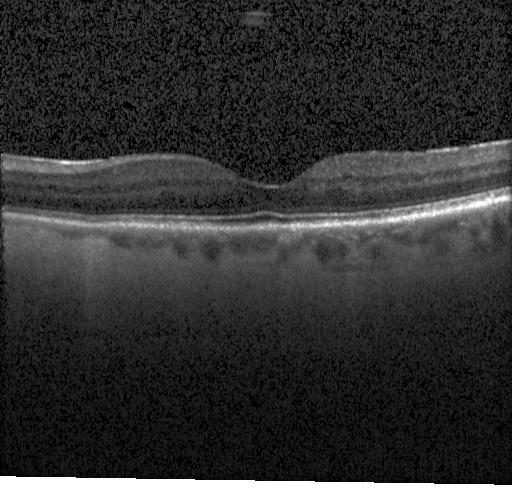
OCT B-scan. Heidelberg Spectralis OCT system. This B-scan demonstrates no CNV, no DME, and no drusen.